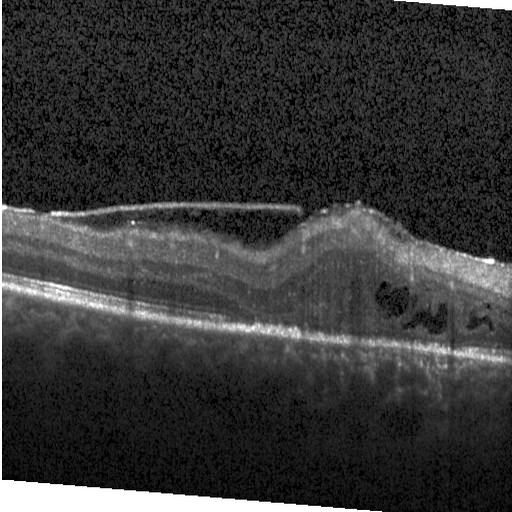
OCT B-scan — Assessment: DME.